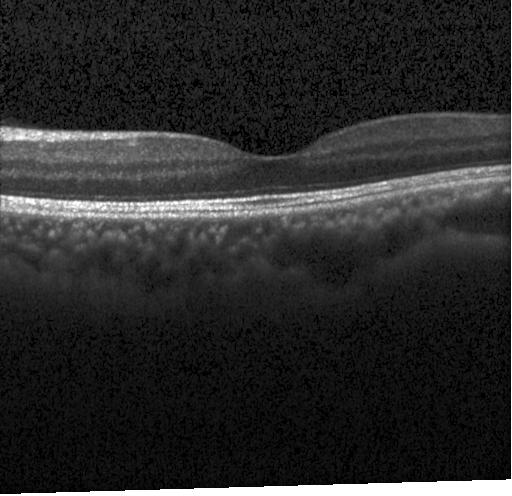
Fovea-centered · OCT line scan · acquired on a Heidelberg Spectralis · SD-OCT. No choroidal neovascularization, no diabetic macular edema, and no drusen.